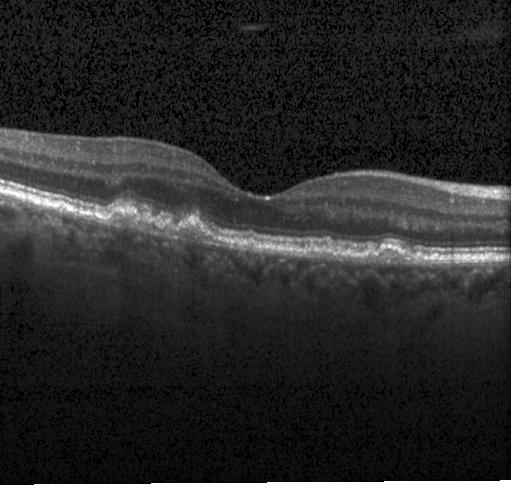
Spectral-domain OCT. Retinal OCT B-scan. Diagnosis: drusen.